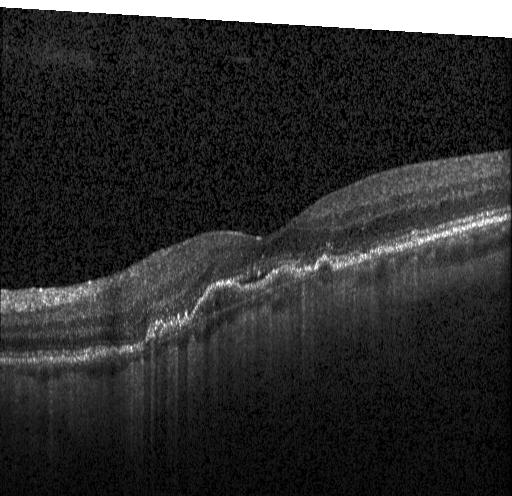
Centered on the fovea; spectral-domain optical coherence tomography; OCT line scan
This B-scan demonstrates choroidal neovascularization.